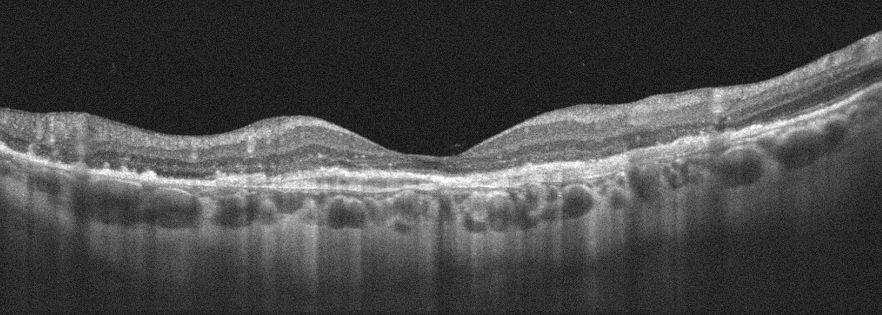

Retinal OCT cross-section, OS — This B-scan demonstrates AMD.